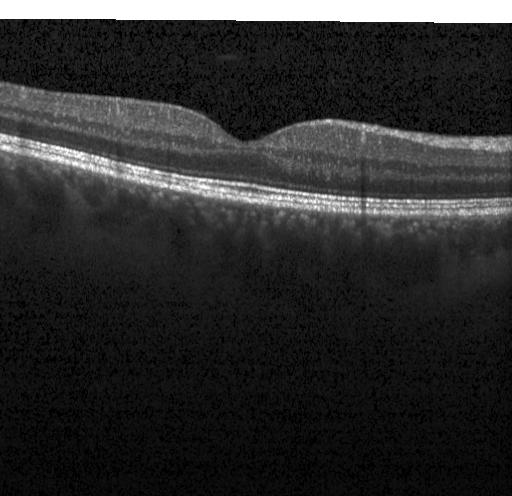 Macular scan; optical coherence tomography scan; spectral-domain optical coherence tomography — Finding: no choroidal neovascularization, no diabetic macular edema, and no drusen.